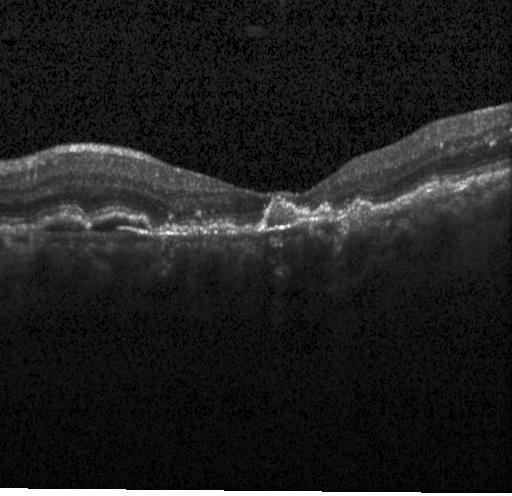 OCT line scan. Finding: choroidal neovascularization.